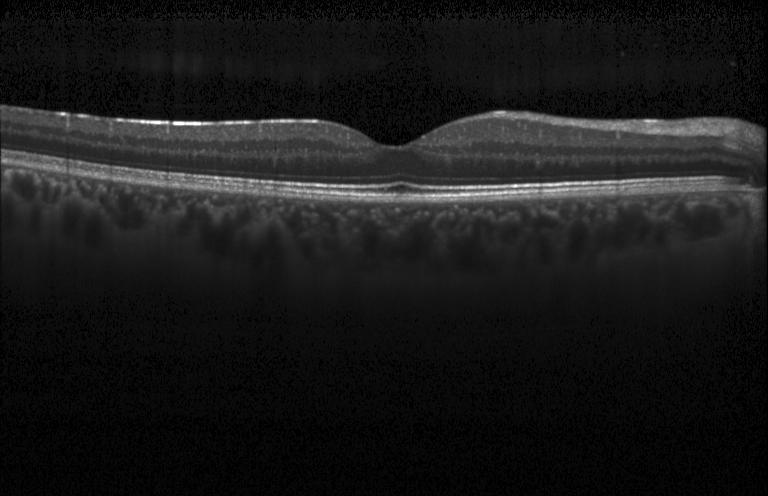
Finding: no CNV, DME, or drusen.